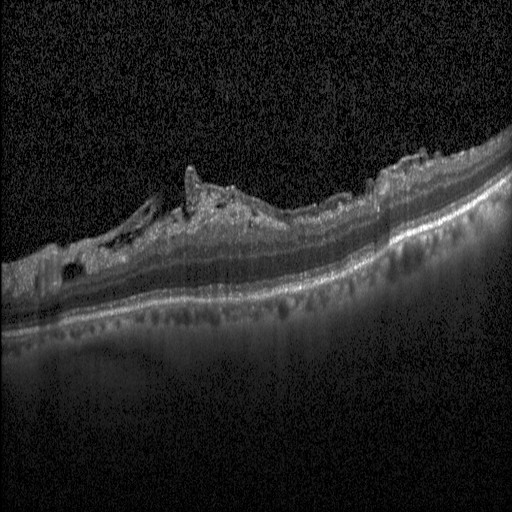
OCT line scan — OCT finding: DME.